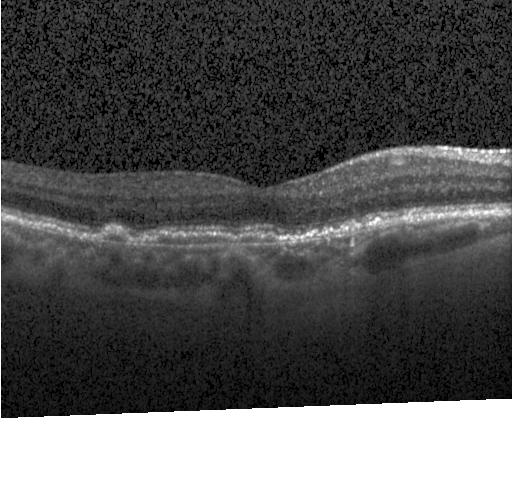

Dx: a choroidal neovascular membrane.